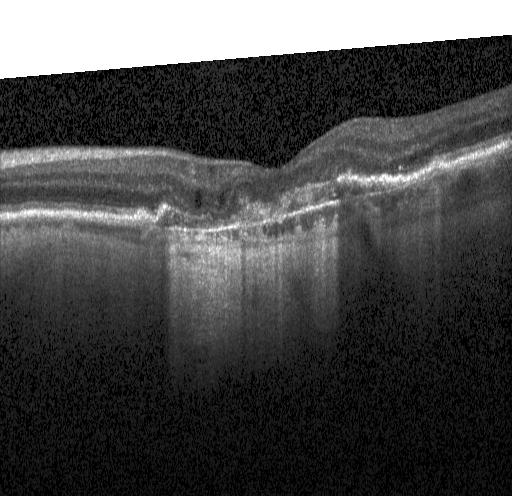 Acquired on a Heidelberg Spectralis · retinal OCT cross-section.
This B-scan demonstrates a choroidal neovascular membrane.